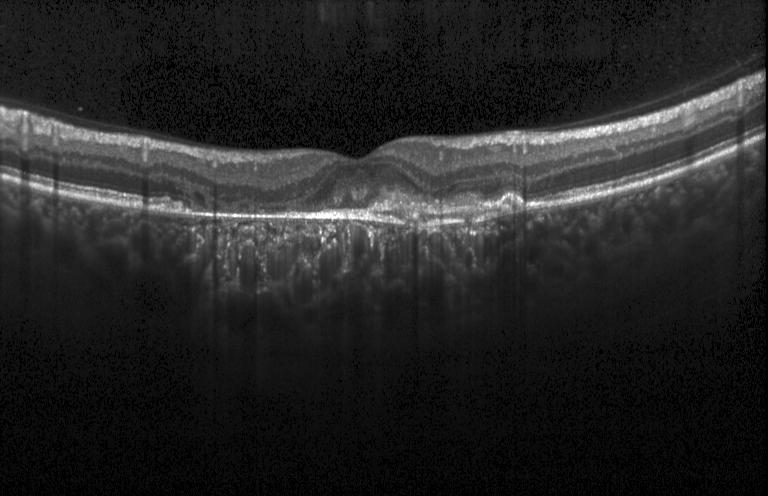 Spectral-domain optical coherence tomography. OCT line scan. Heidelberg Spectralis — Finding: choroidal neovascularization (CNV).